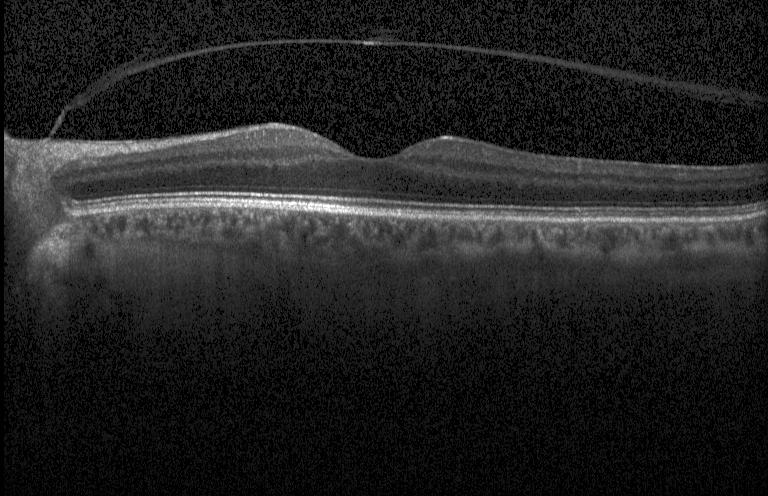
Retinal OCT B-scan, SD-OCT, Heidelberg Spectralis OCT system, fovea-centered.
Assessment: neither choroidal neovascularization, diabetic macular edema, nor drusen.